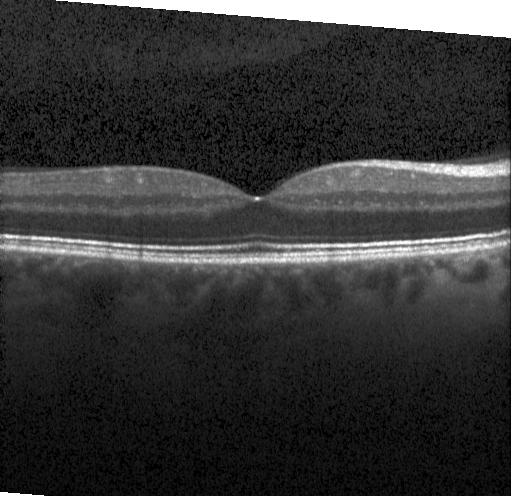

Spectral-domain OCT; retinal OCT cross-section; through the macula; acquired on a Heidelberg Spectralis. Diagnosis: neither choroidal neovascularization, diabetic macular edema, nor drusen.